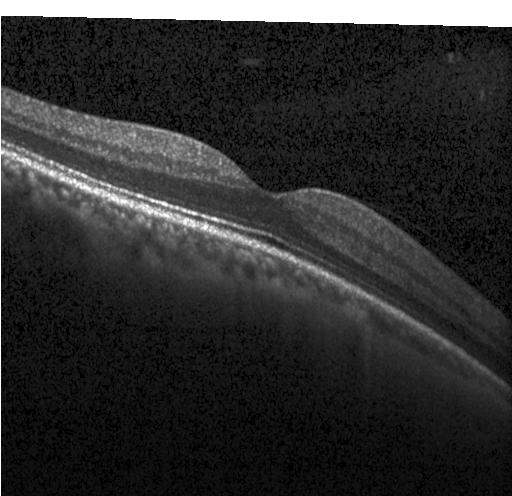
Spectral-domain optical coherence tomography; retinal OCT B-scan; centered on the fovea. OCT finding: neither choroidal neovascularization, diabetic macular edema, nor drusen.